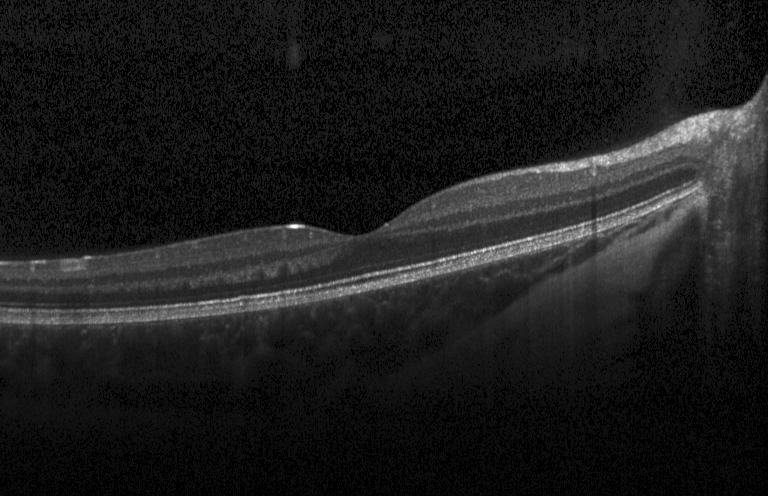

OCT line scan, through the macula, SD-OCT, Heidelberg Spectralis OCT system — Diagnosis: no choroidal neovascularization, no diabetic macular edema, and no drusen.